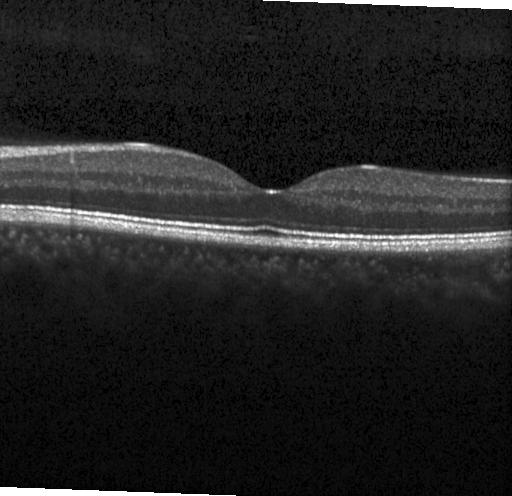
OCT line scan; SD-OCT; Heidelberg Spectralis OCT system; horizontal scan through the fovea.
Diagnosis: no choroidal neovascularization, no diabetic macular edema, and no drusen.